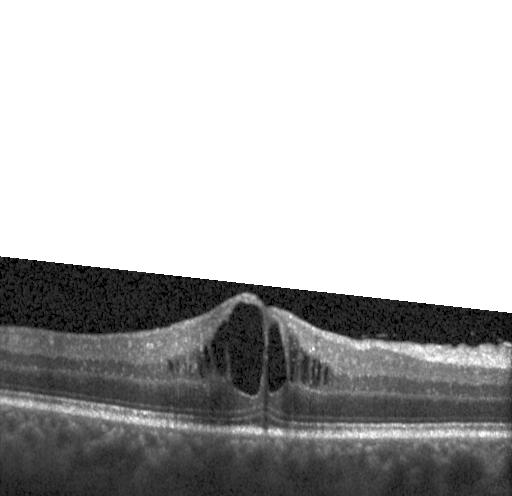
Acquired on a Heidelberg Spectralis; macular scan; optical coherence tomography B-scan
Impression: diabetic macular edema.